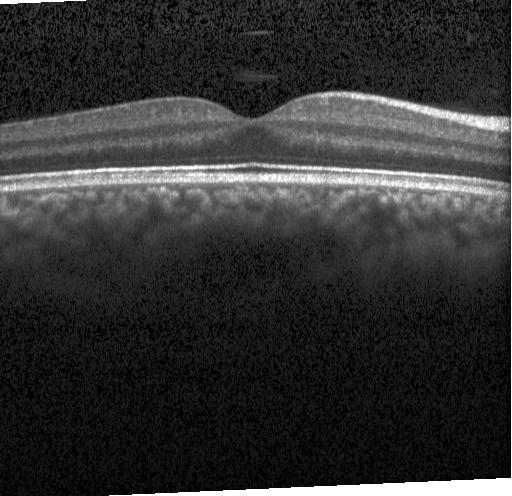
Retinal OCT B-scan; instrument: Heidelberg Spectralis.
Impression: no evidence of choroidal neovascularization, diabetic macular edema, or drusen.